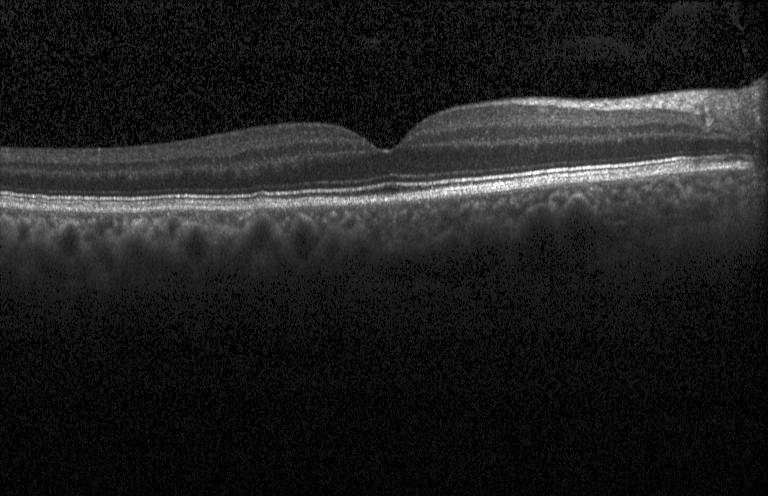

Optical coherence tomography scan; instrument: Heidelberg Spectralis
This B-scan demonstrates no choroidal neovascularization, diabetic macular edema, or drusen.